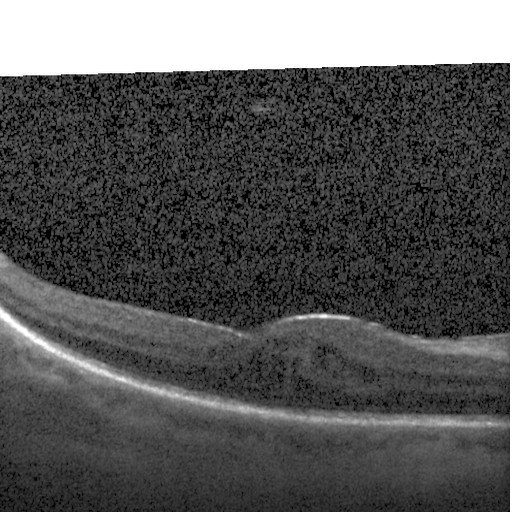

Retinal OCT cross-section, fovea-centered.
Diagnosis: diabetic macular edema.